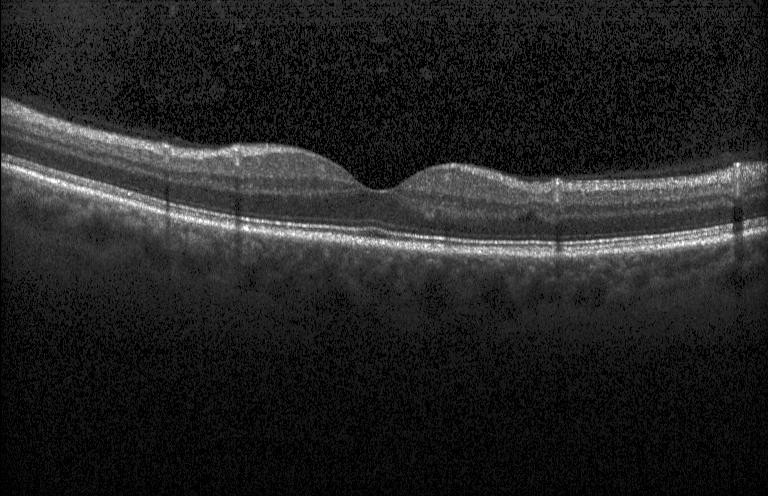
Impression: no choroidal neovascularization, no diabetic macular edema, and no drusen.